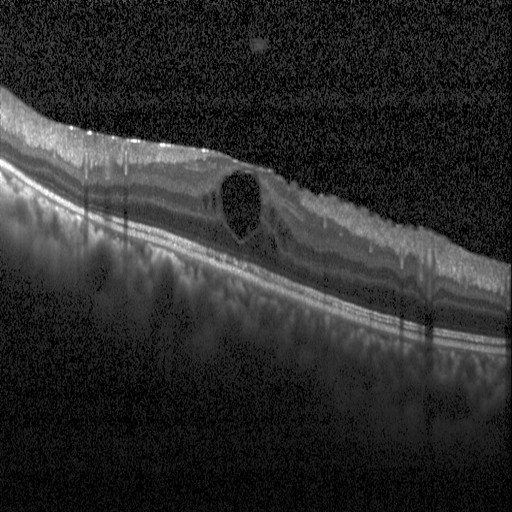 OCT scan showing diabetic macular edema.